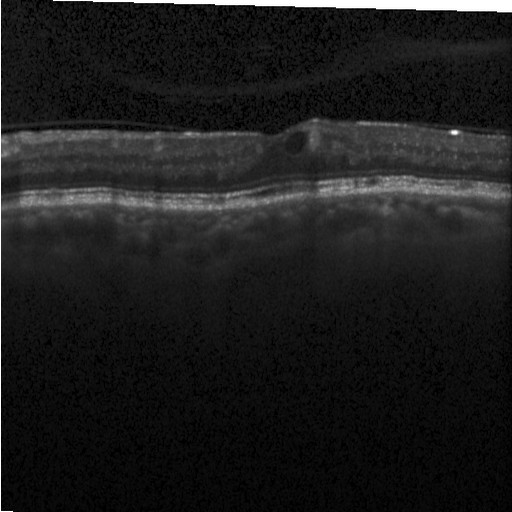
Horizontal scan through the fovea, spectral-domain optical coherence tomography, optical coherence tomography scan, acquired on a Heidelberg Spectralis.
Diagnosis: DME.